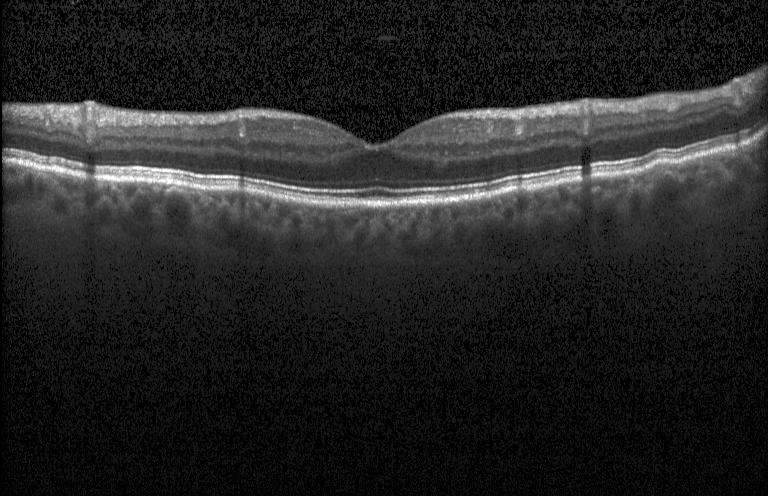

Dx: neither CNV, DME, nor drusen.